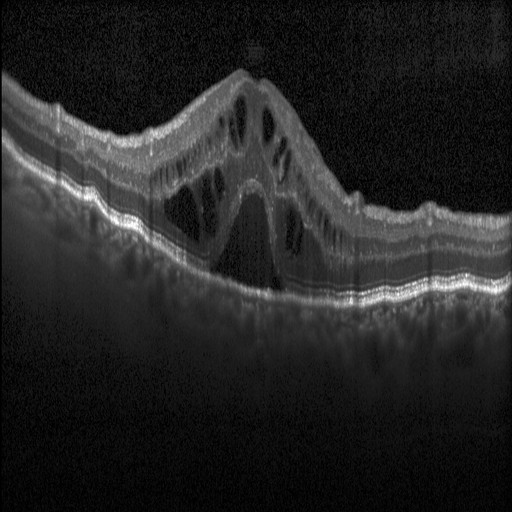
Retinal OCT B-scan
This B-scan demonstrates diabetic macular edema.